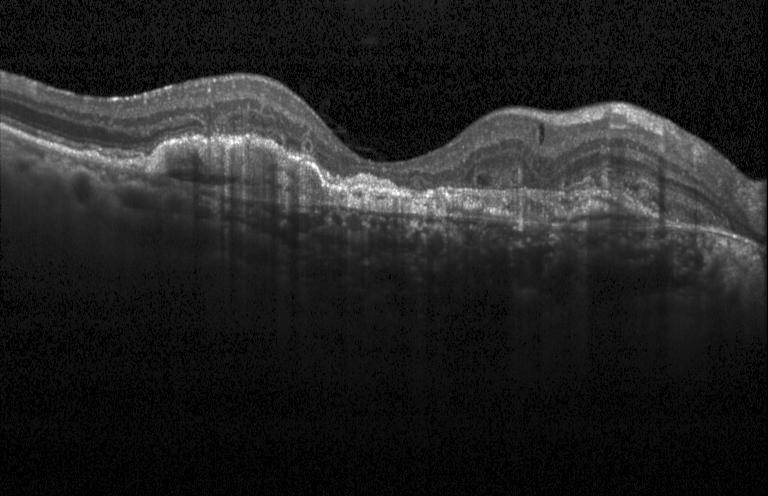

Optical coherence tomography scan · acquired on a Heidelberg Spectralis · spectral-domain OCT.
Diagnosis: choroidal neovascularization (CNV).